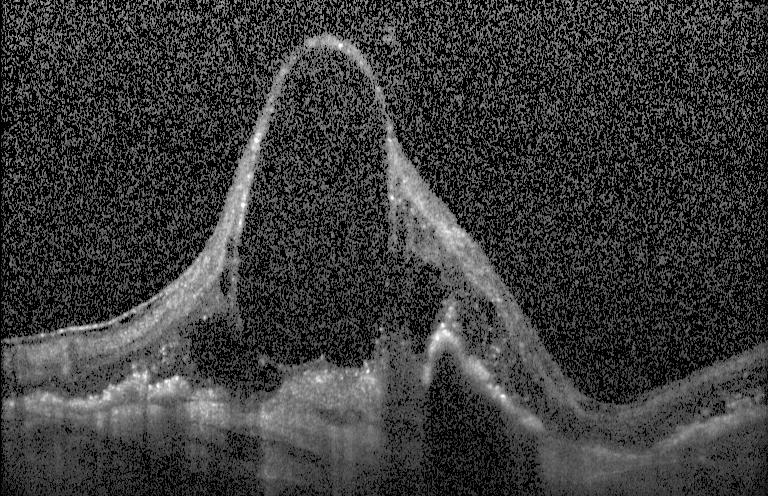
SD-OCT; OCT B-scan
Assessment: choroidal neovascularization.